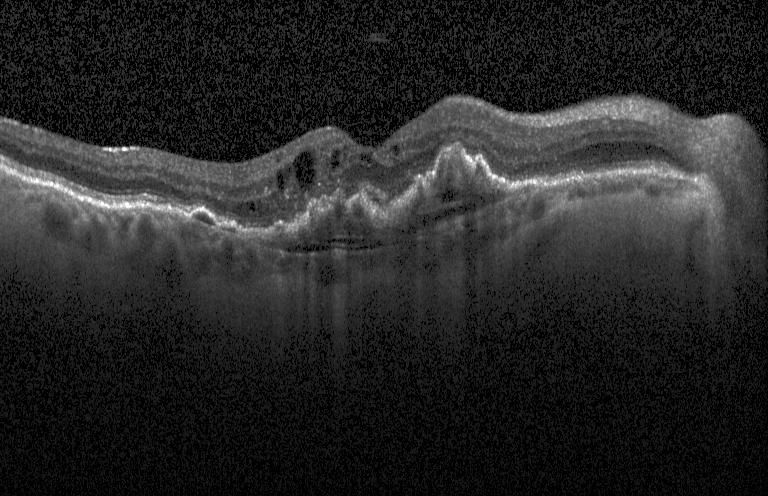

Finding: CNV.